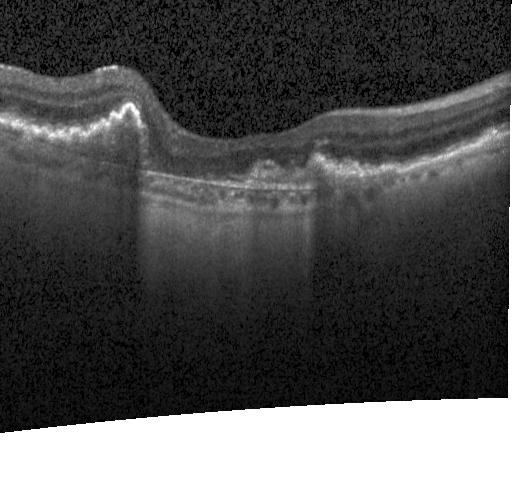
Retinal OCT cross-section showing choroidal neovascularization.